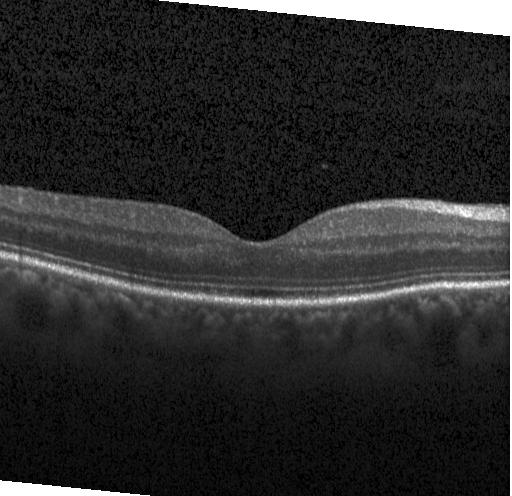

Diagnosis: neither CNV, DME, nor drusen.